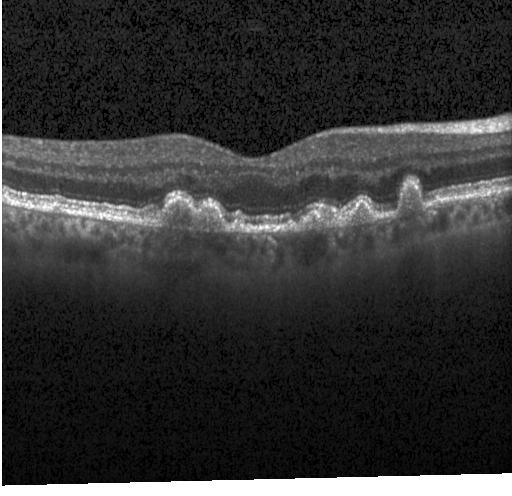 Optical coherence tomography B-scan
Impression: multiple drusen.